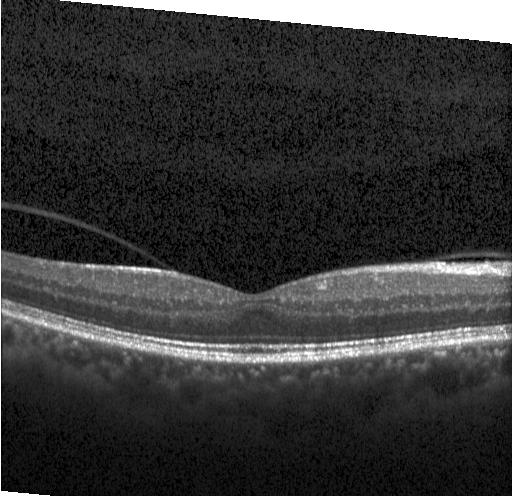 Optical coherence tomography scan. Impression: no evidence of choroidal neovascularization, diabetic macular edema, or drusen.